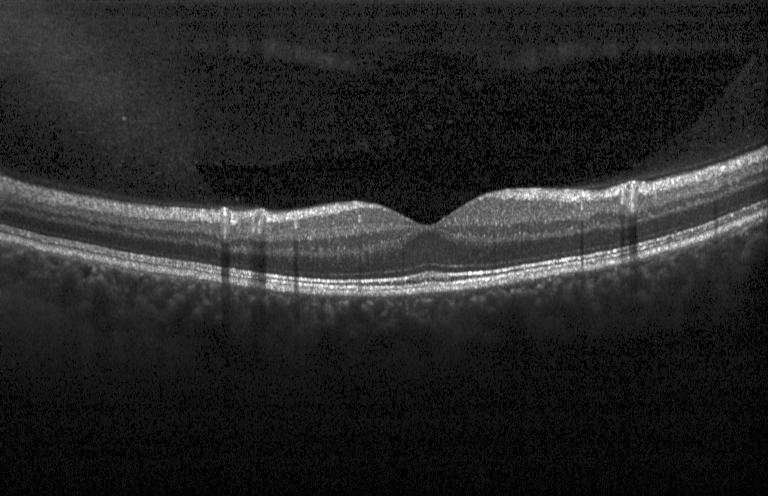
Retinal OCT cross-section.
Macular OCT: no CNV, no DME, and no drusen.